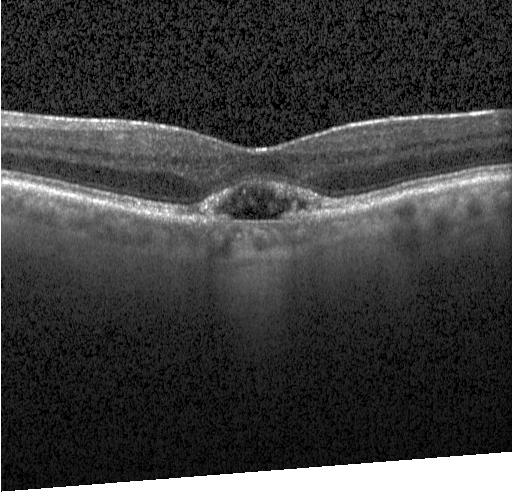 Spectral-domain OCT B-scan: a choroidal neovascular membrane.